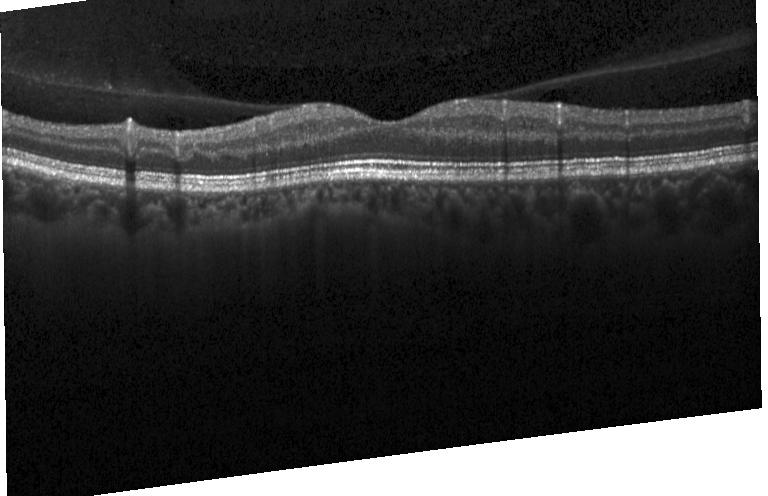

OCT B-scan.
Diagnosis: no choroidal neovascularization, no diabetic macular edema, and no drusen.